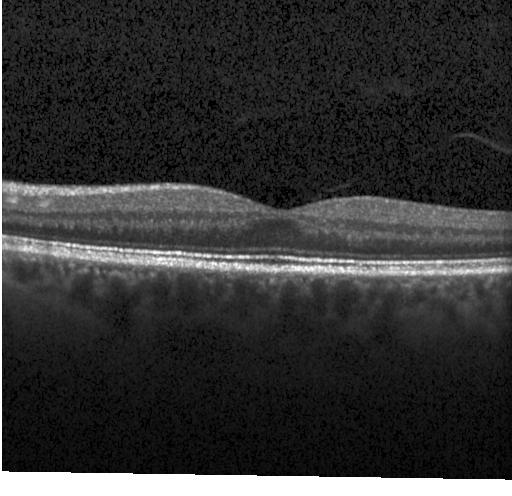
Diagnosis: no choroidal neovascularization, diabetic macular edema, or drusen.